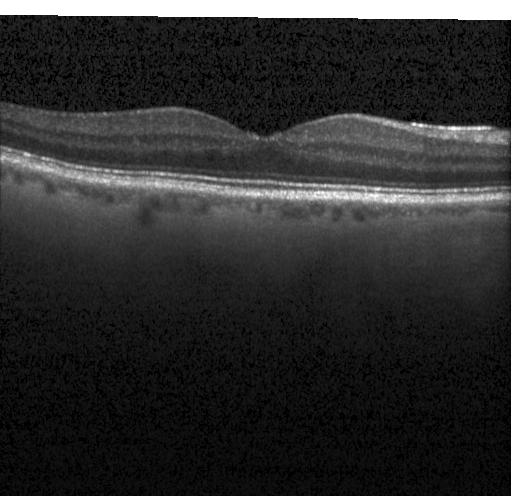

Optical coherence tomography B-scan; macular scan — Finding: no choroidal neovascularization, no diabetic macular edema, and no drusen.